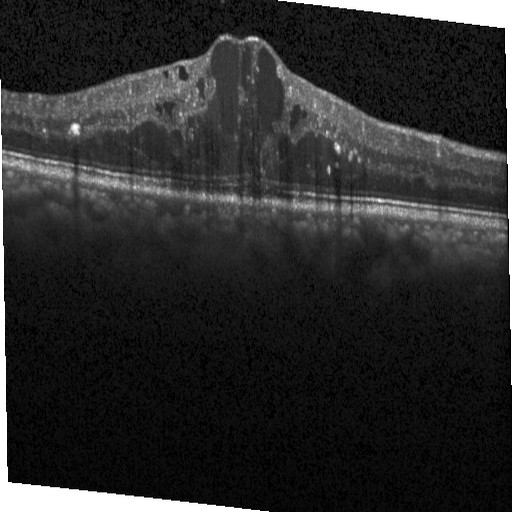 Retinal OCT B-scan. This B-scan demonstrates diabetic macular edema.